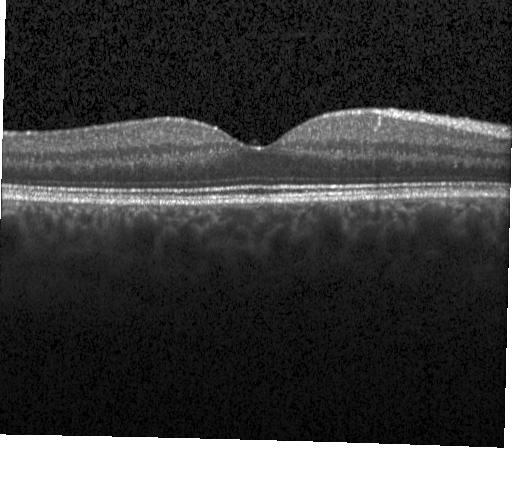

Spectral-domain OCT. Heidelberg Spectralis OCT system. Retinal OCT B-scan
Diagnosis: no CNV, no DME, and no drusen.